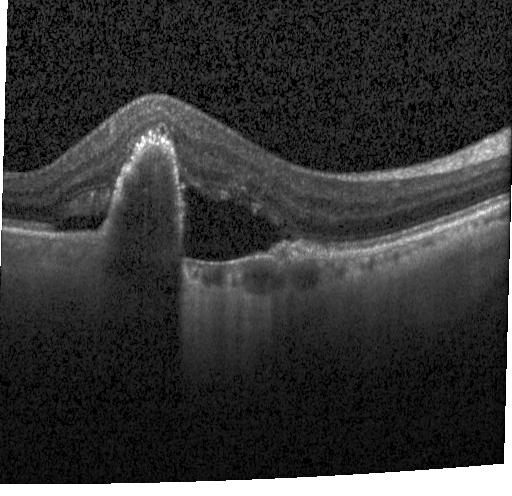

OCT line scan.
Finding: choroidal neovascularization (CNV).